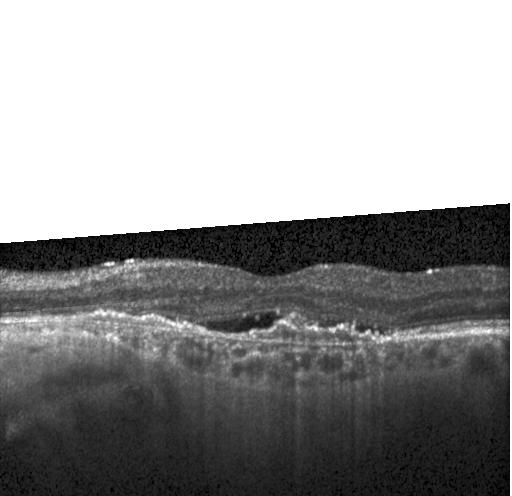 Retinal OCT cross-section showing a choroidal neovascular membrane.